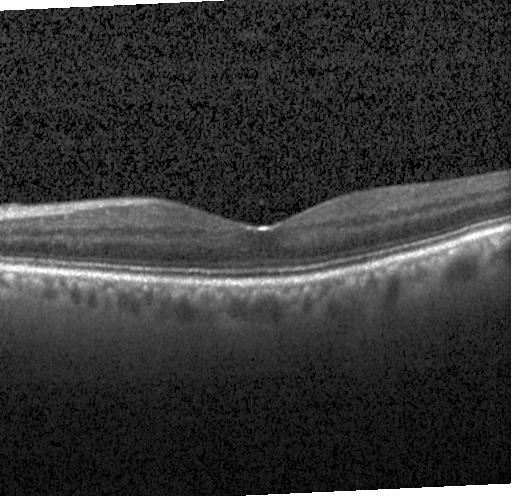
Optical coherence tomography scan · spectral-domain optical coherence tomography. Finding: no CNV, DME, or drusen.